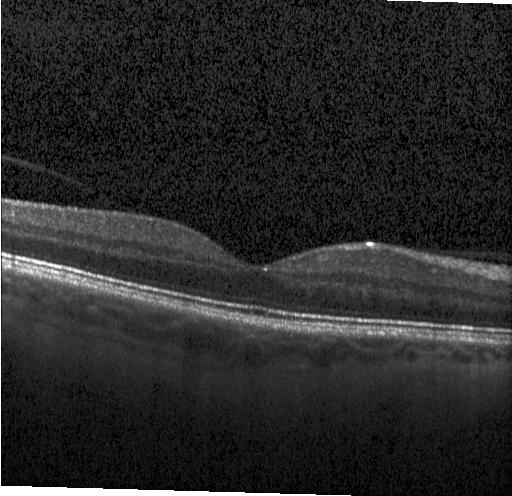 Retinal OCT B-scan, spectral-domain optical coherence tomography, Heidelberg Spectralis OCT system.
Assessment: no evidence of CNV, DME, or drusen.